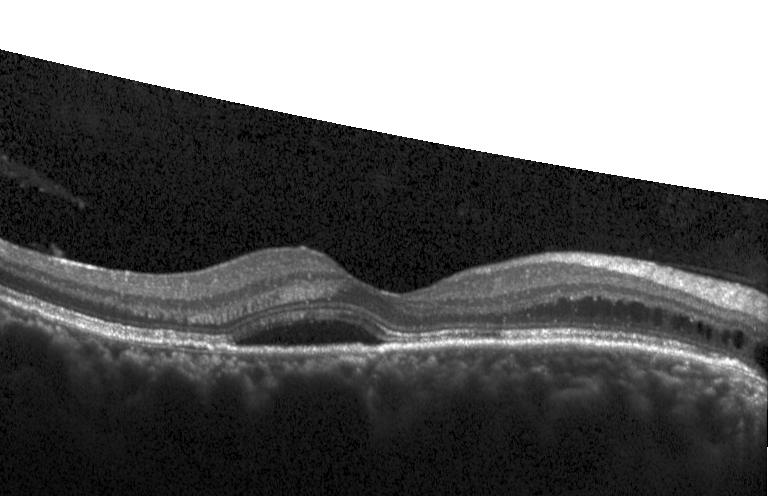

Finding: choroidal neovascularization.